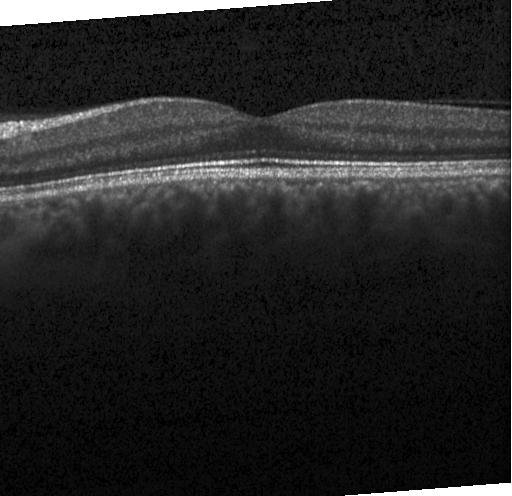
Finding: no choroidal neovascularization, no diabetic macular edema, and no drusen.